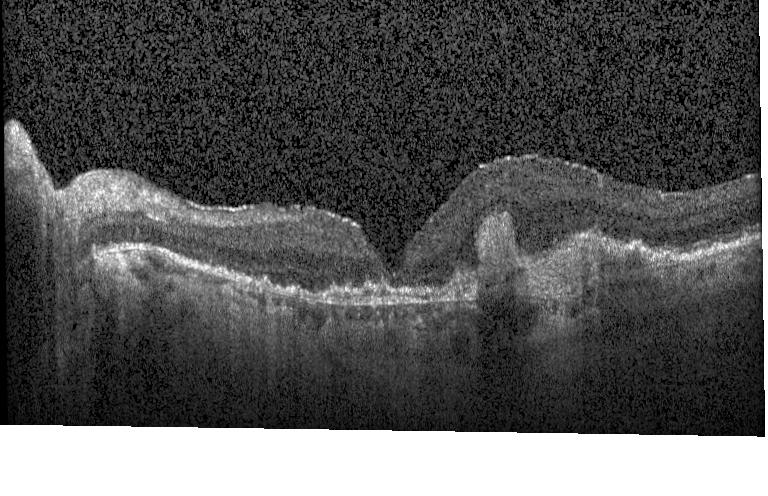
Optical coherence tomography scan, spectral-domain optical coherence tomography.
Impression: CNV.